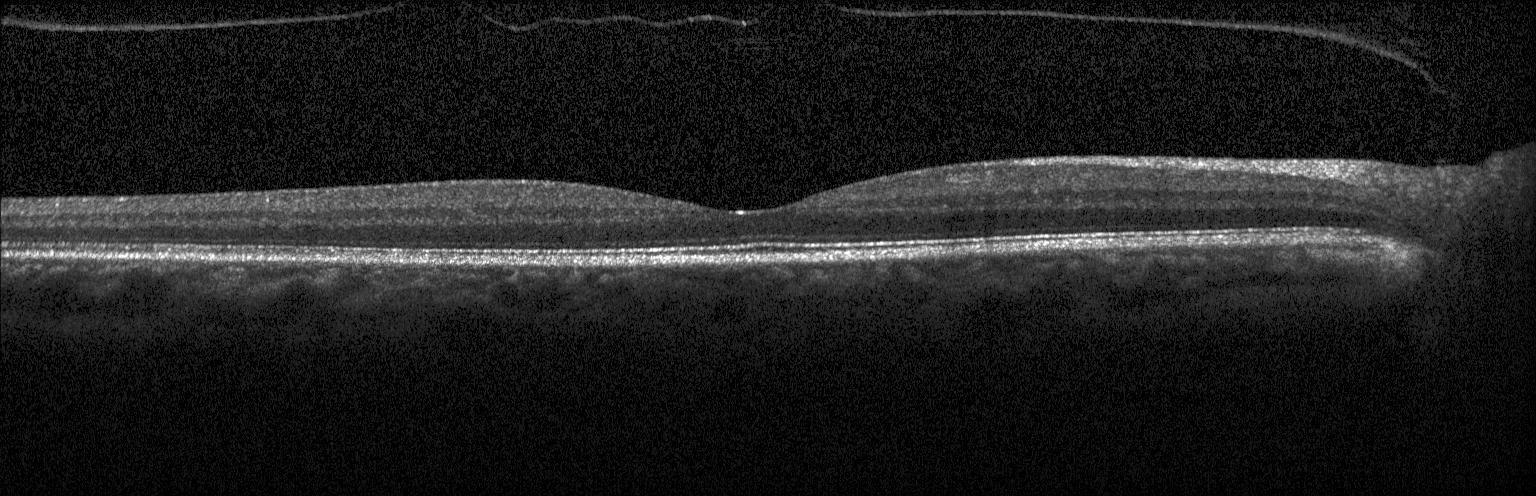 Spectral-domain optical coherence tomography · macular scan · retinal OCT B-scan · instrument: Heidelberg Spectralis
No CNV, no DME, and no drusen.